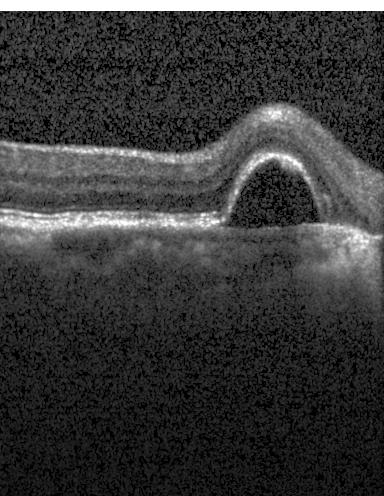 Optical coherence tomography scan — Finding: a choroidal neovascular membrane.